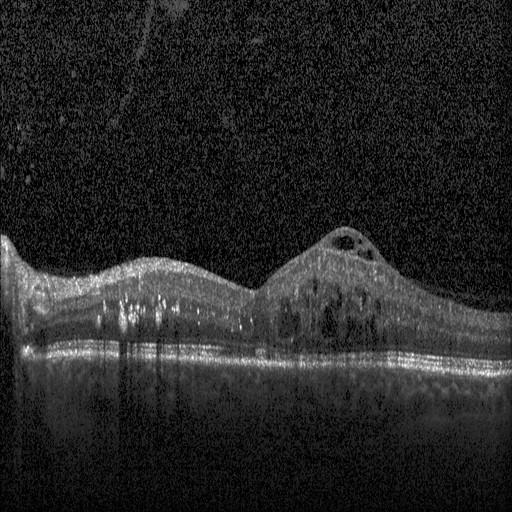
This B-scan demonstrates DME.